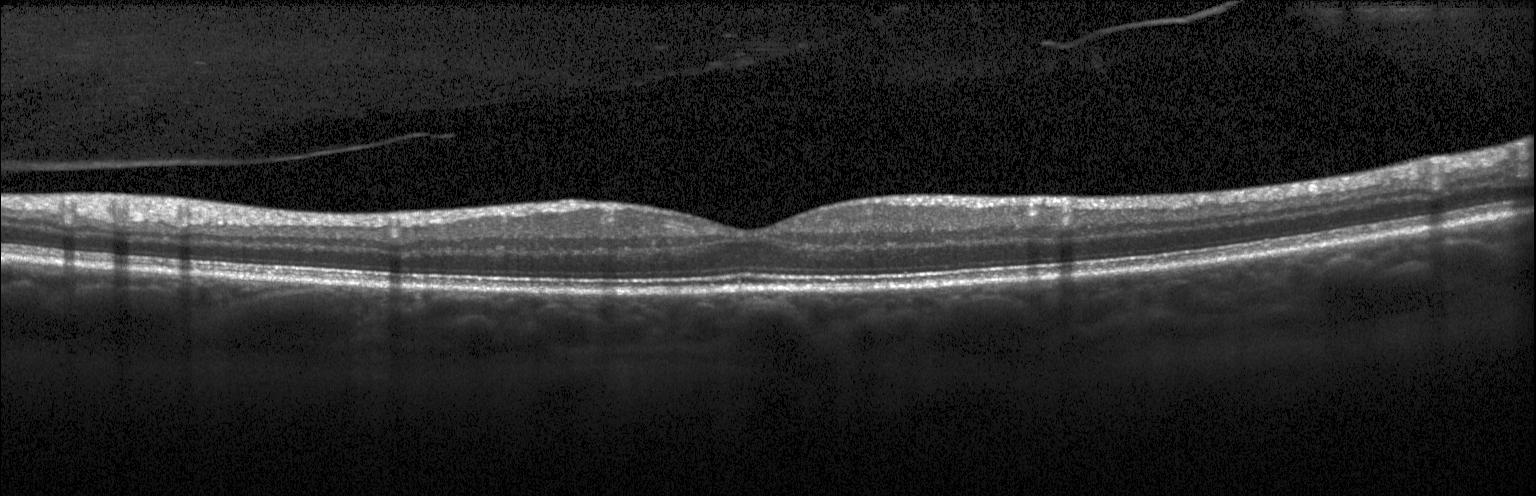 OCT finding: no choroidal neovascularization, diabetic macular edema, or drusen.